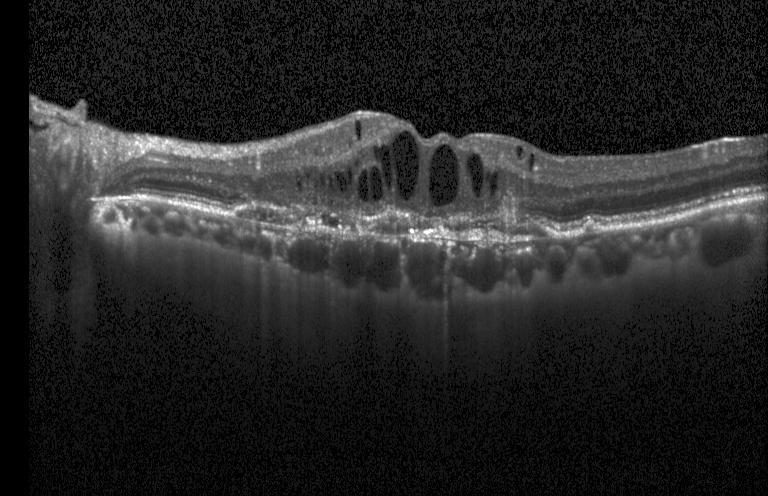

Retinal OCT B-scan. Assessment: choroidal neovascularization.